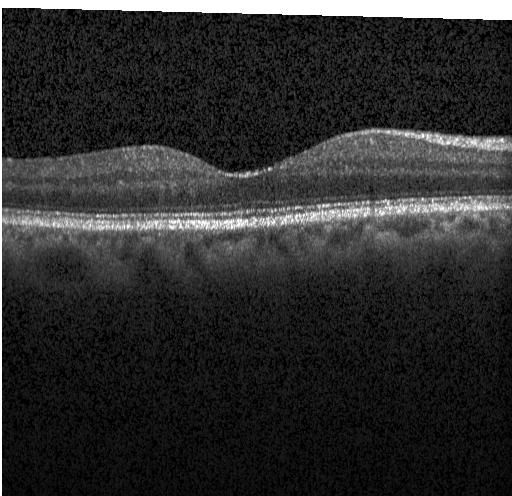

Acquired on a Heidelberg Spectralis · spectral-domain OCT · optical coherence tomography B-scan
Dx: neither choroidal neovascularization, diabetic macular edema, nor drusen.